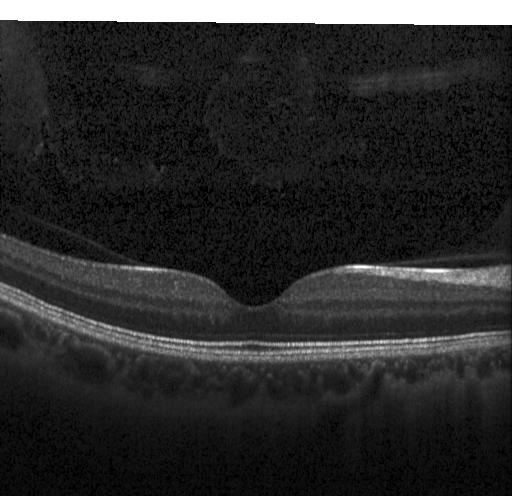 OCT B-scan. Centered on the fovea. Heidelberg Spectralis.
Diagnosis: neither choroidal neovascularization, diabetic macular edema, nor drusen.